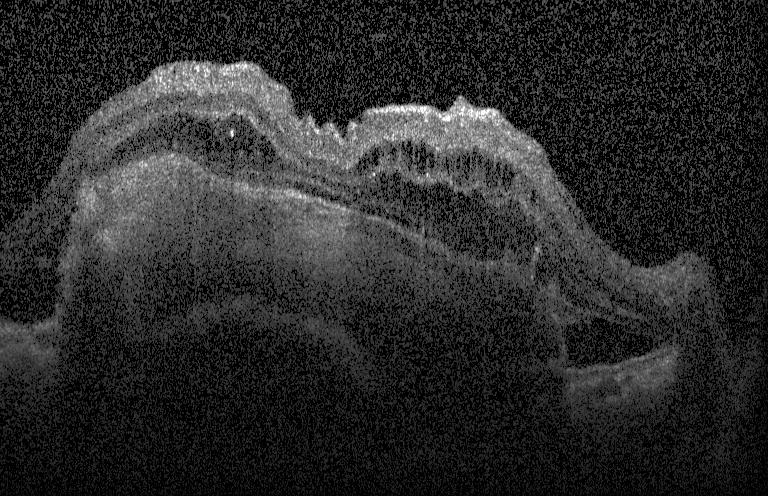 Dx: a choroidal neovascular membrane.